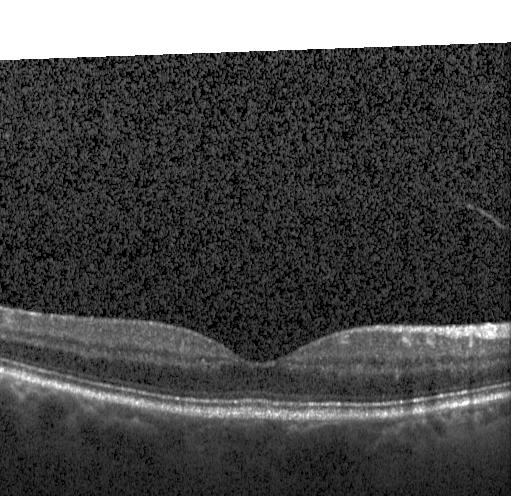 Optical coherence tomography scan, through the macula, spectral-domain OCT.
Macular OCT: no CNV, no DME, and no drusen.